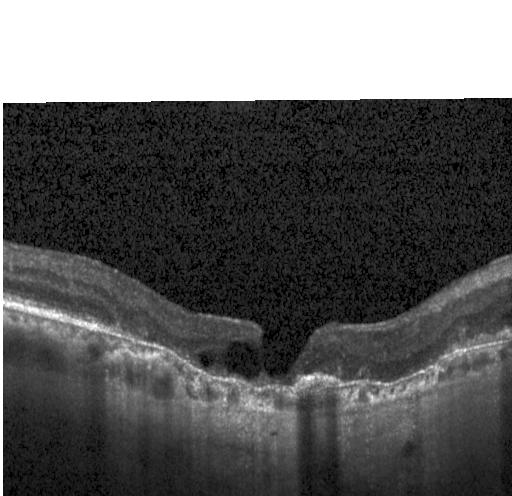

Spectral-domain OCT; retinal OCT B-scan — Assessment: choroidal neovascularization.